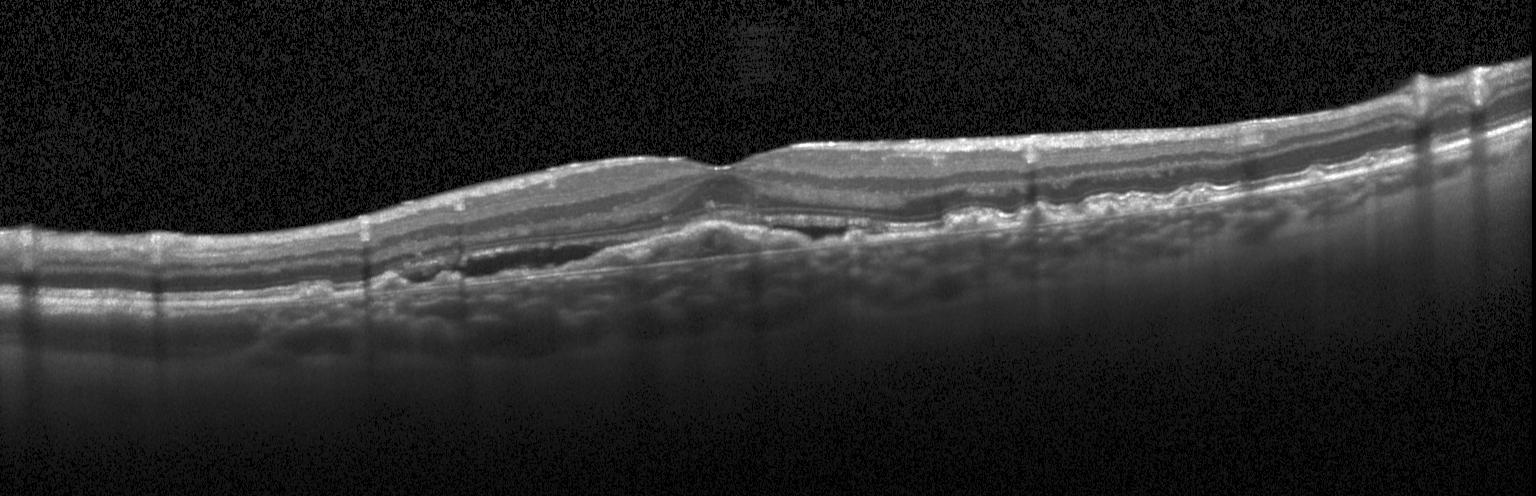
OCT B-scan, SD-OCT, fovea-centered. Assessment: choroidal neovascularization (CNV).